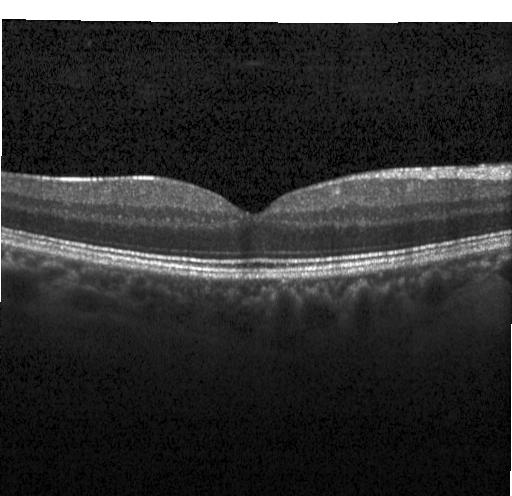
Horizontal scan through the fovea. Heidelberg Spectralis OCT system. Optical coherence tomography B-scan
Finding: no evidence of CNV, DME, or drusen.